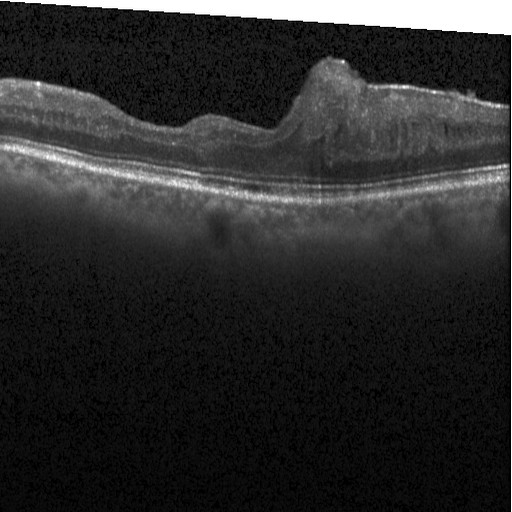

OCT B-scan · spectral-domain optical coherence tomography.
OCT finding: diabetic macular edema (DME).